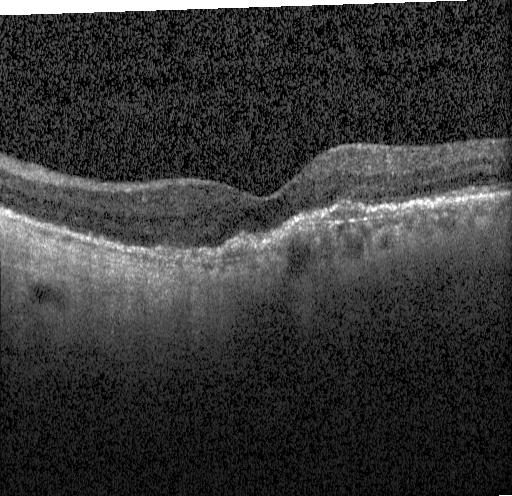
Spectral-domain OCT · acquired on a Heidelberg Spectralis · macular scan · retinal OCT B-scan. This B-scan demonstrates choroidal neovascularization (CNV).